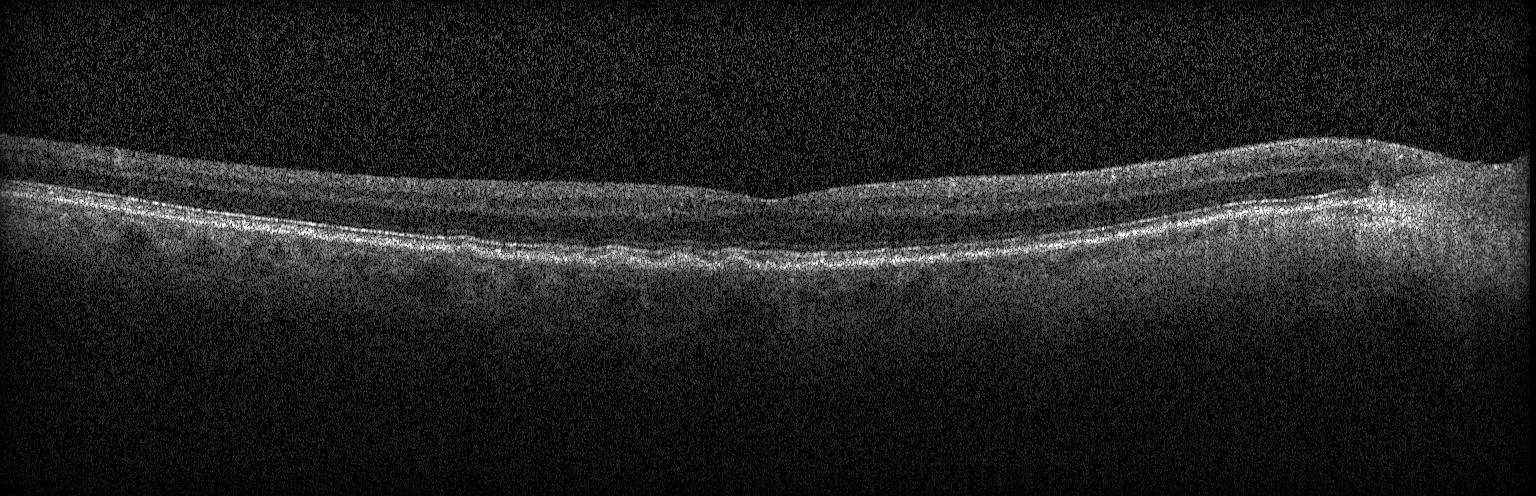
OCT line scan. Finding: multiple drusen.